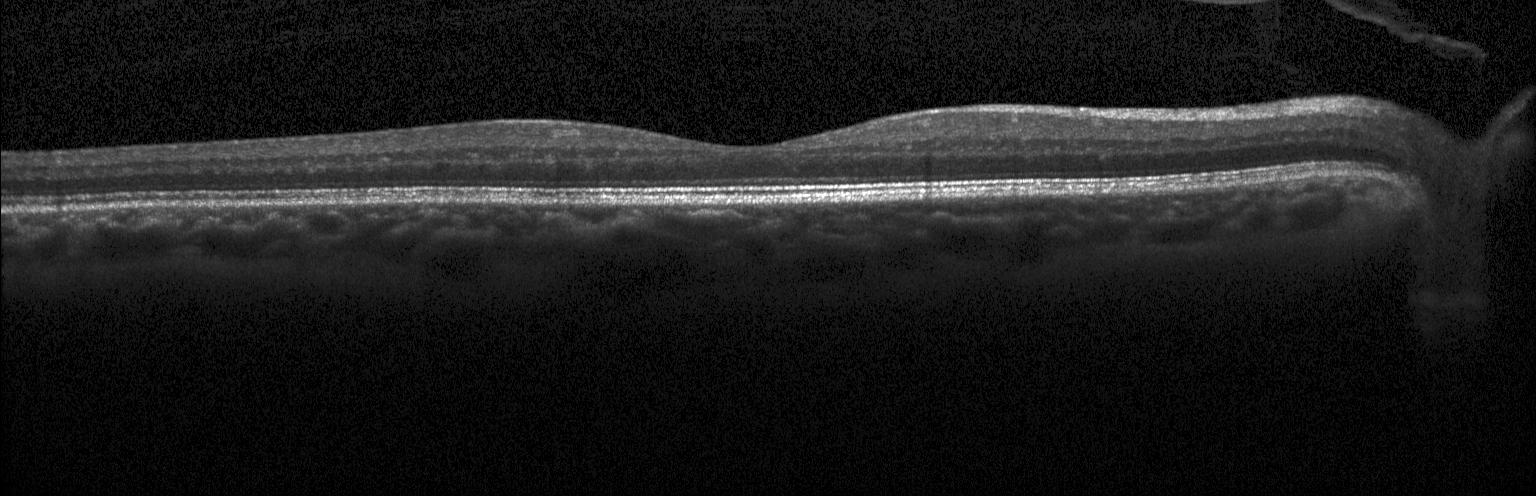 SD-OCT; OCT B-scan; through the macula; acquired on a Heidelberg Spectralis.
Finding: neither choroidal neovascularization, diabetic macular edema, nor drusen.